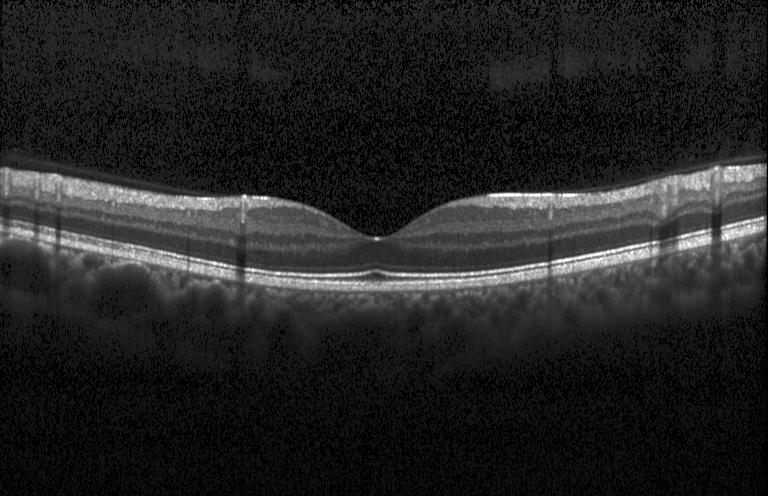

Horizontal scan through the fovea. Retinal OCT B-scan. Acquired on a Heidelberg Spectralis.
Finding: no choroidal neovascularization, no diabetic macular edema, and no drusen.